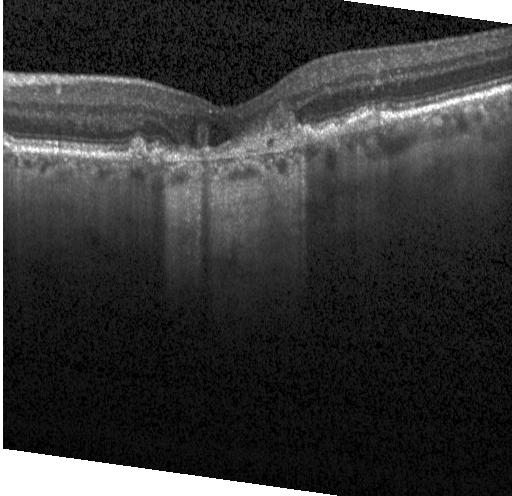 OCT line scan. Horizontal scan through the fovea — Finding: CNV.